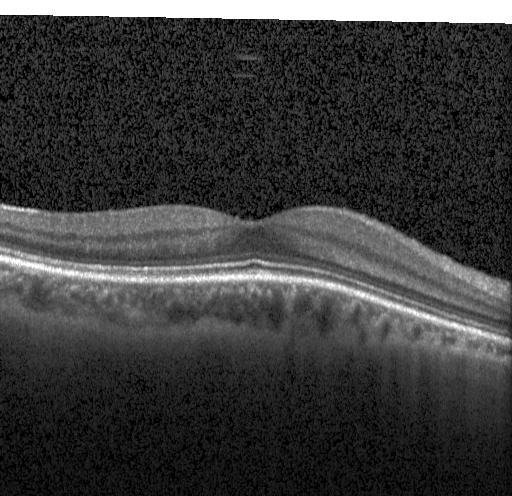 Finding: no choroidal neovascularization, no diabetic macular edema, and no drusen.